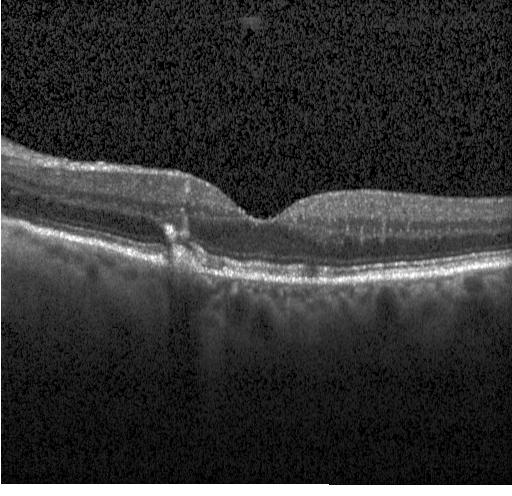
Heidelberg Spectralis OCT system · horizontal scan through the fovea · OCT line scan
Diagnosis: multiple drusen.